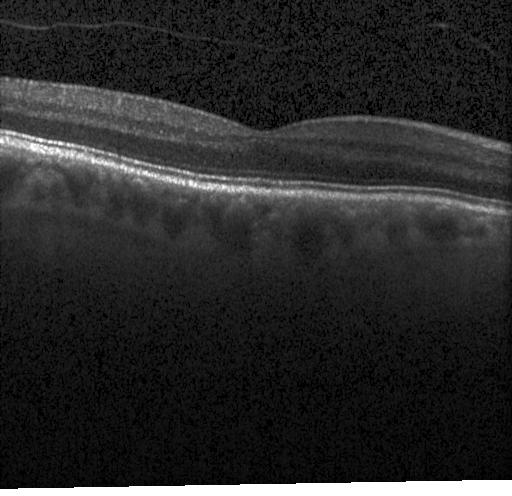

Through the macula; SD-OCT; Heidelberg Spectralis OCT system; OCT line scan
Assessment: neither choroidal neovascularization, diabetic macular edema, nor drusen.